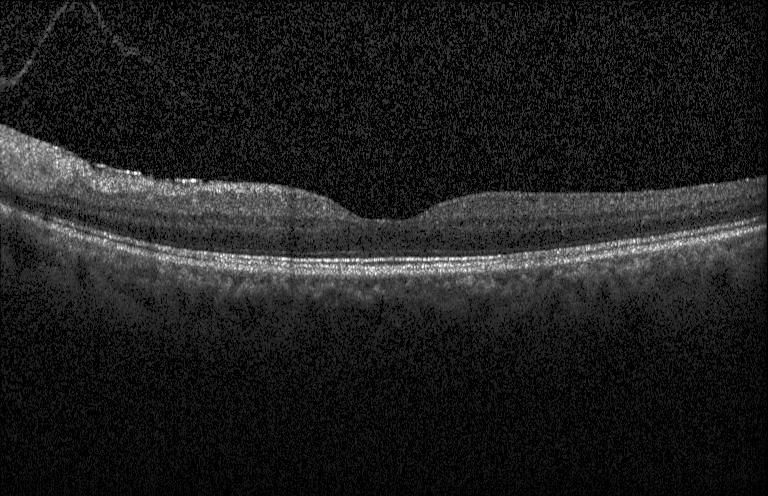
Spectral-domain optical coherence tomography, acquired on a Heidelberg Spectralis, optical coherence tomography scan.
Finding: no CNV, no DME, and no drusen.